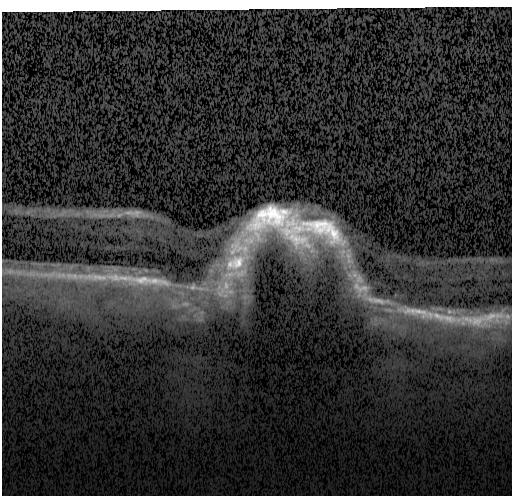
Optical coherence tomography B-scan — Assessment: choroidal neovascularization (CNV).